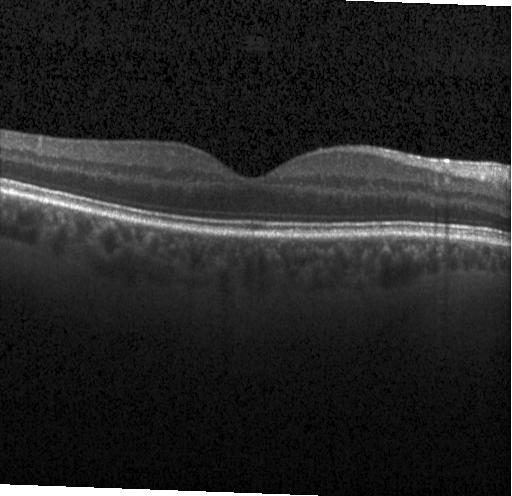
OCT scan showing no choroidal neovascularization, diabetic macular edema, or drusen.